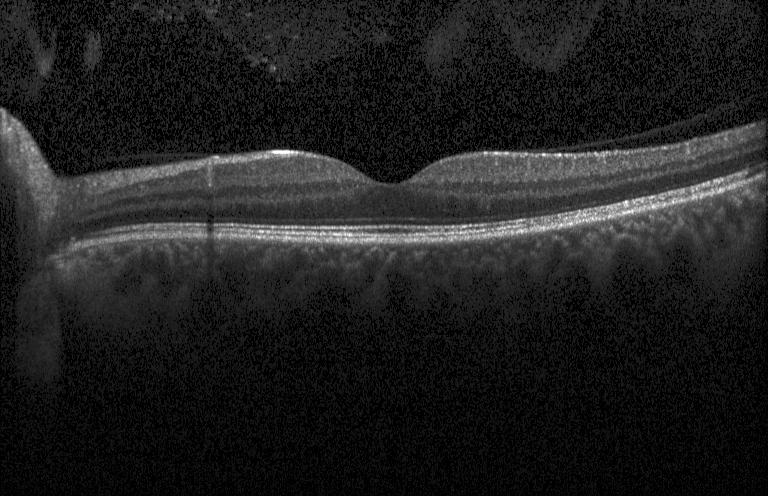 Retinal OCT cross-section
Impression: no choroidal neovascularization, diabetic macular edema, or drusen.